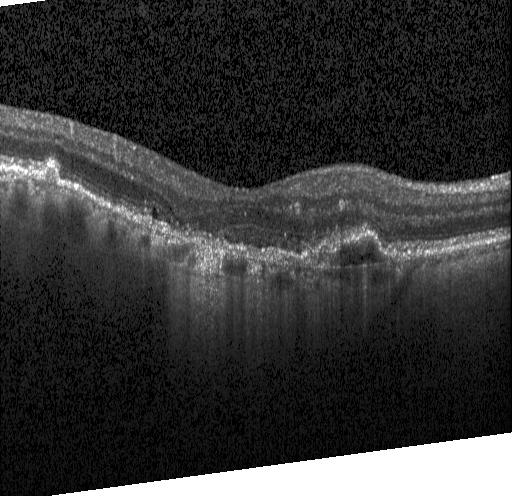

OCT B-scan. Finding: a choroidal neovascular membrane.